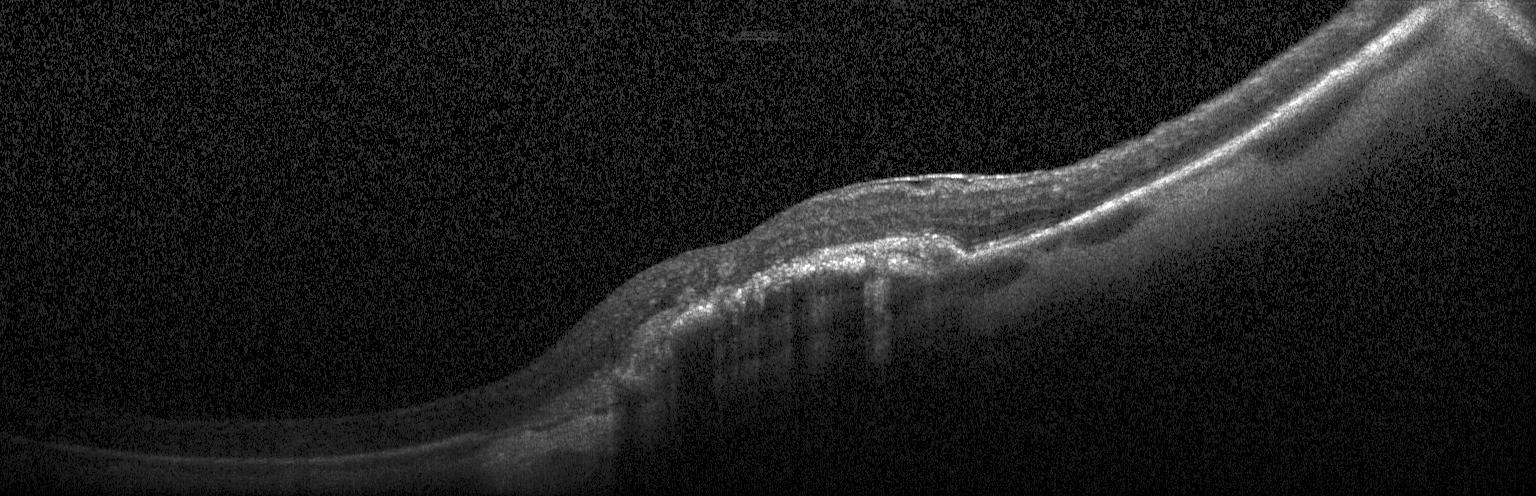
Retinal OCT B-scan
Diagnosis: choroidal neovascularization.